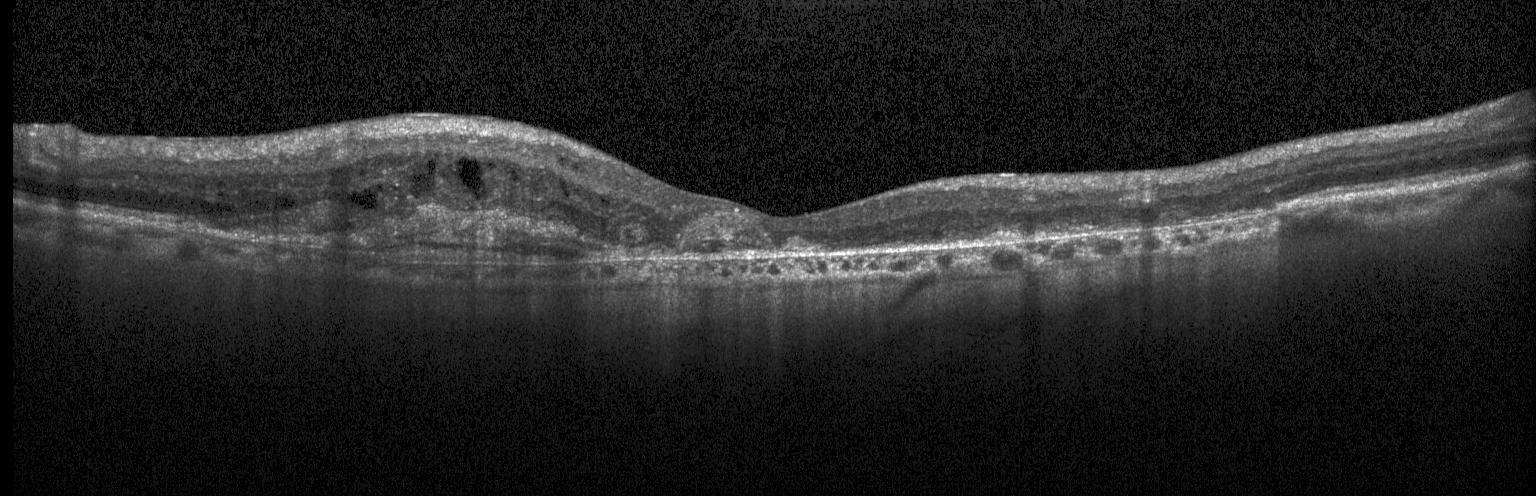 Retinal OCT B-scan; acquired on a Heidelberg Spectralis; spectral-domain optical coherence tomography.
Assessment: choroidal neovascularization.